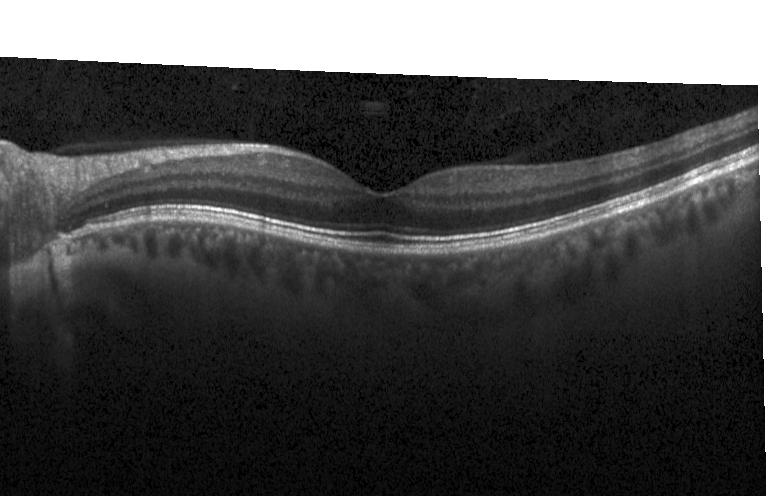 Impression: no CNV, no DME, and no drusen.